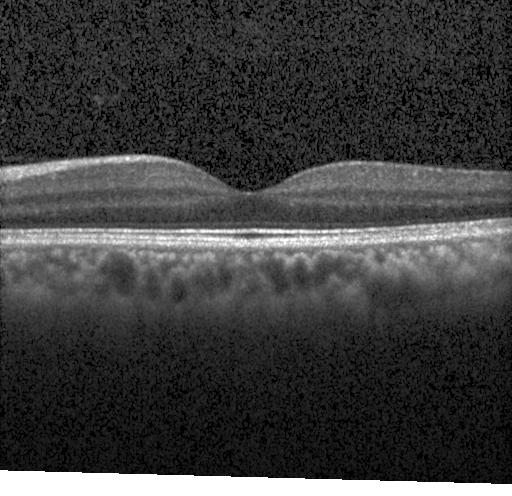

Spectral-domain OCT B-scan: no CNV, DME, or drusen.